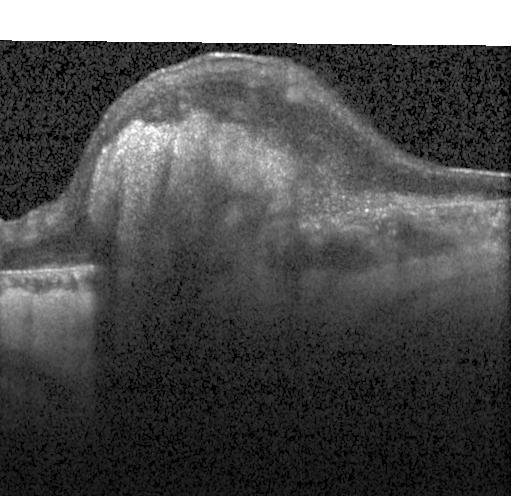
Retinal OCT cross-section. Choroidal neovascularization (CNV).